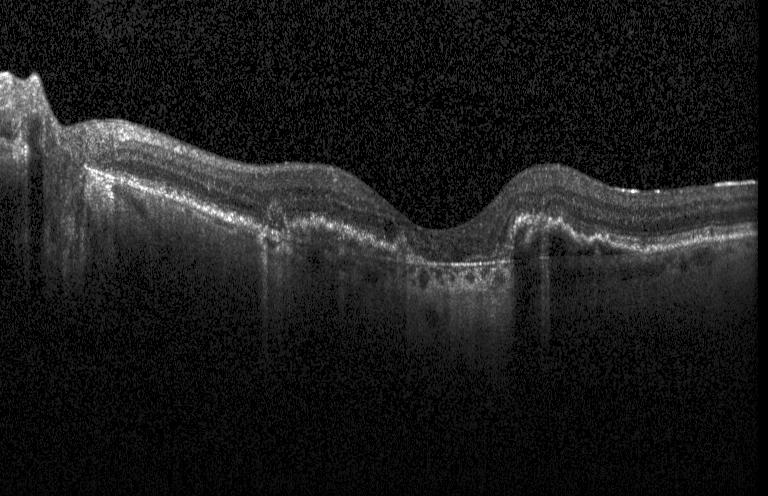 Through the macula; SD-OCT; acquired on a Heidelberg Spectralis; retinal OCT B-scan
Diagnosis: a choroidal neovascular membrane.